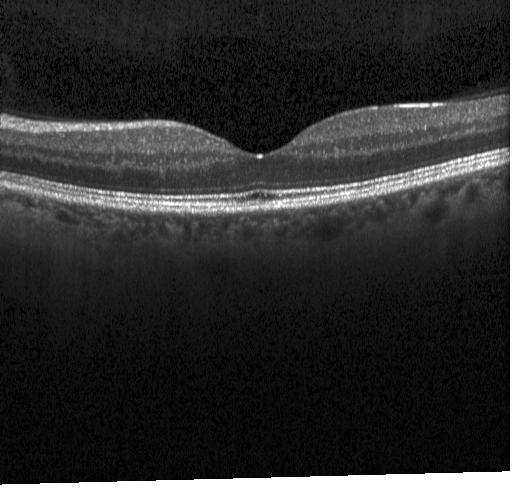 OCT scan showing no evidence of choroidal neovascularization, diabetic macular edema, or drusen.